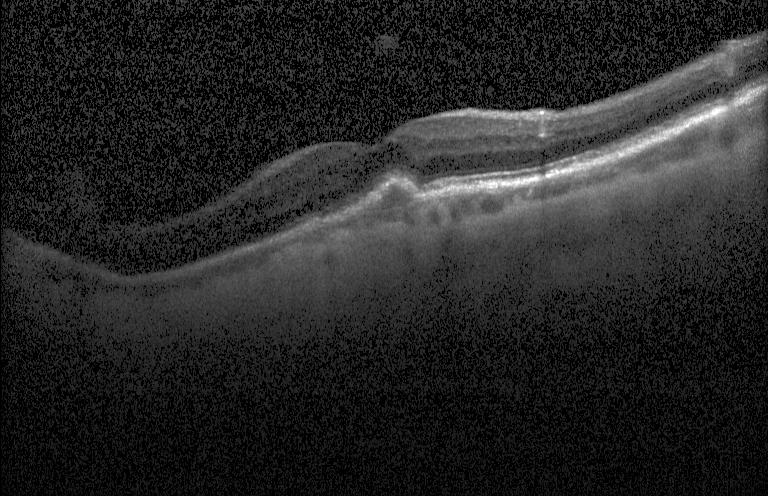 Optical coherence tomography B-scan, spectral-domain OCT. This B-scan demonstrates sub-RPE drusenoid deposits.